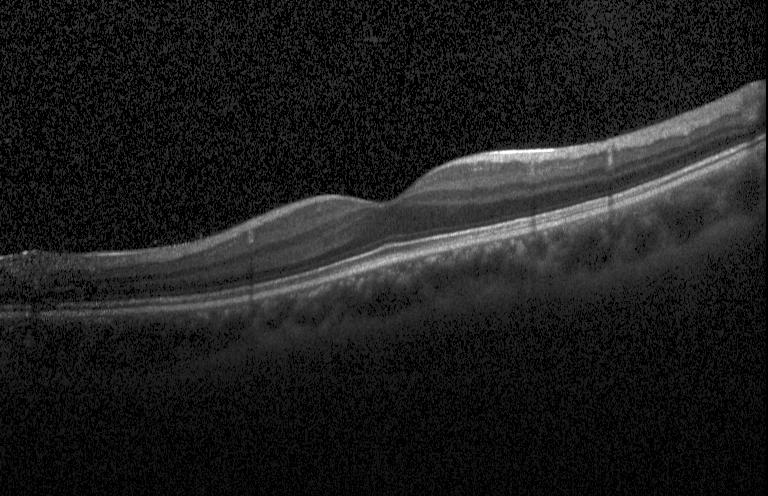
Diagnosis: no evidence of CNV, DME, or drusen.